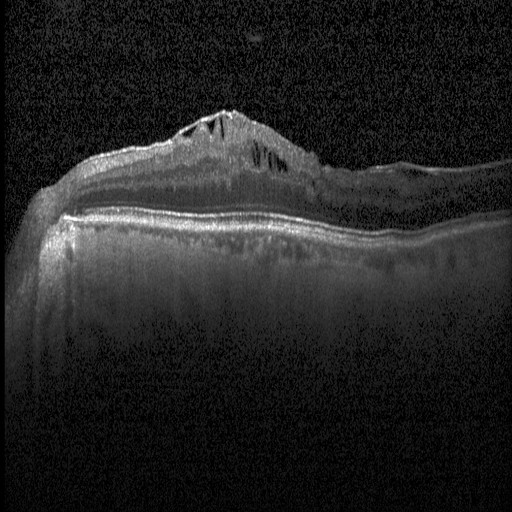 Diabetic macular edema.